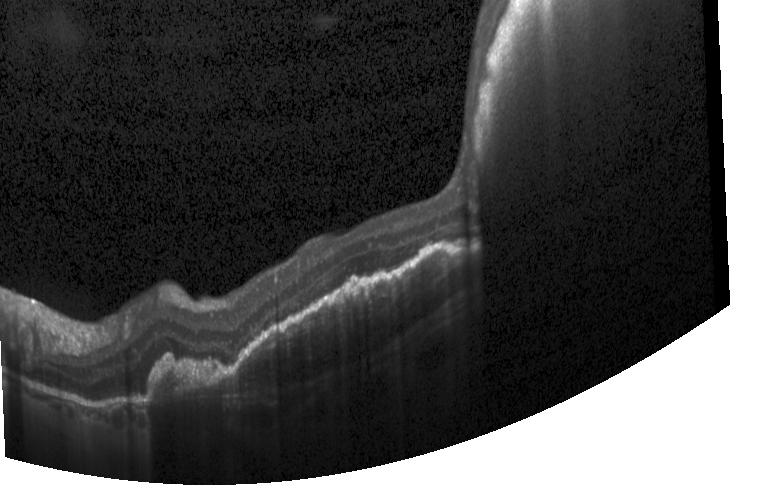

Diagnosis: a choroidal neovascular membrane.